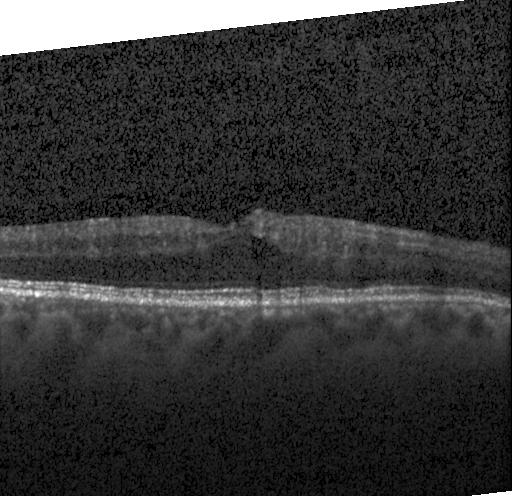 Retinal OCT cross-section. Finding: DME.